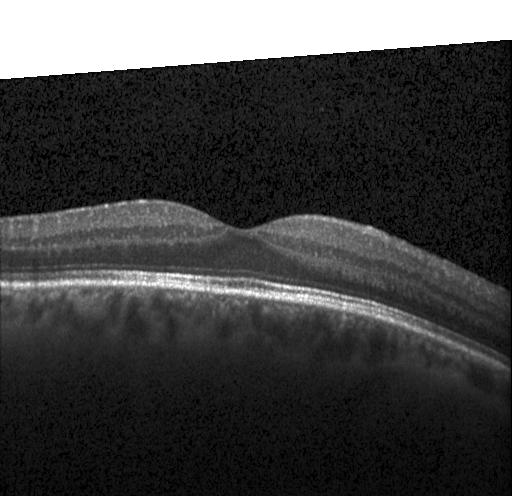
Horizontal scan through the fovea · spectral-domain optical coherence tomography · Heidelberg Spectralis · optical coherence tomography scan — Diagnosis: no evidence of choroidal neovascularization, diabetic macular edema, or drusen.